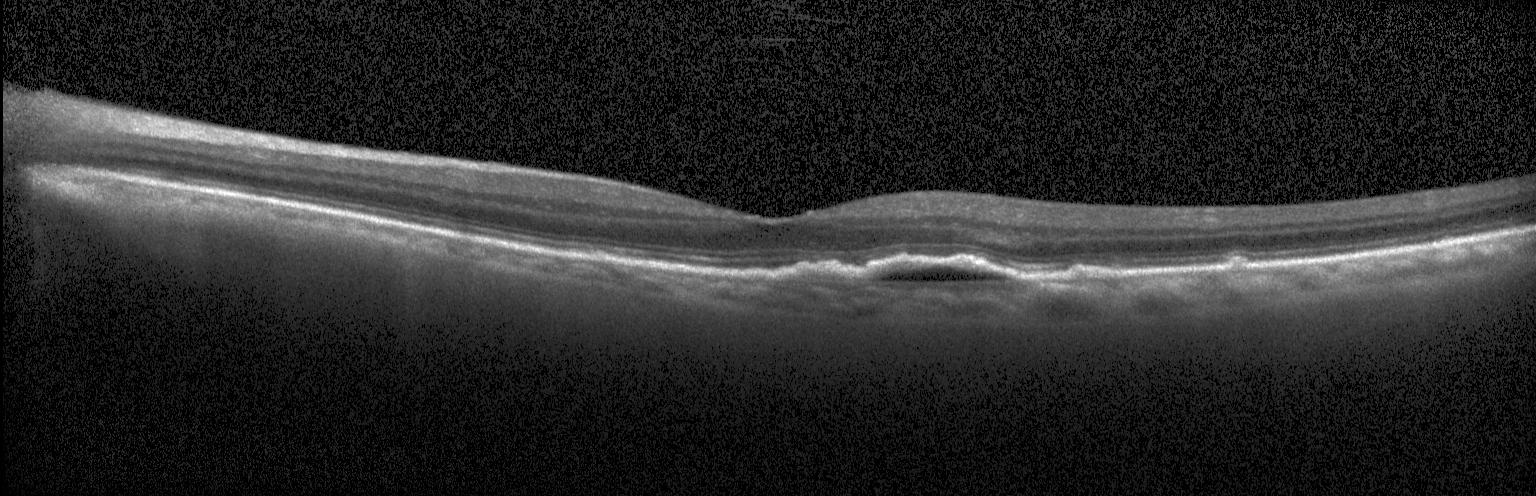
Impression: CNV.